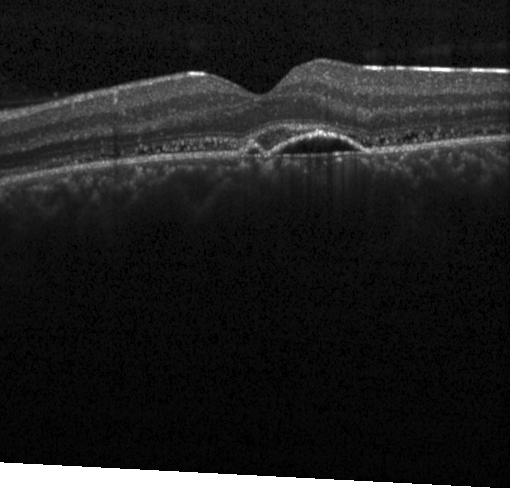
Fovea-centered · retinal OCT cross-section · spectral-domain optical coherence tomography · acquired on a Heidelberg Spectralis.
Choroidal neovascularization.